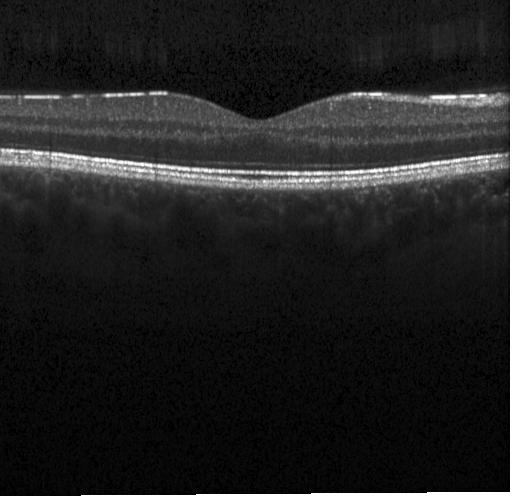
Optical coherence tomography B-scan; acquired on a Heidelberg Spectralis; through the macula; spectral-domain OCT
Assessment: no choroidal neovascularization, no diabetic macular edema, and no drusen.